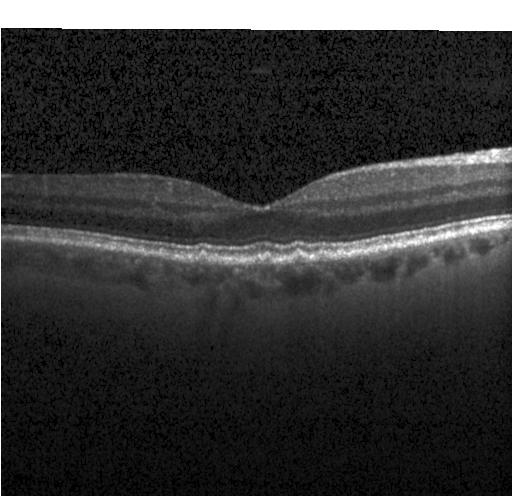 OCT line scan
This B-scan demonstrates sub-RPE drusenoid deposits.